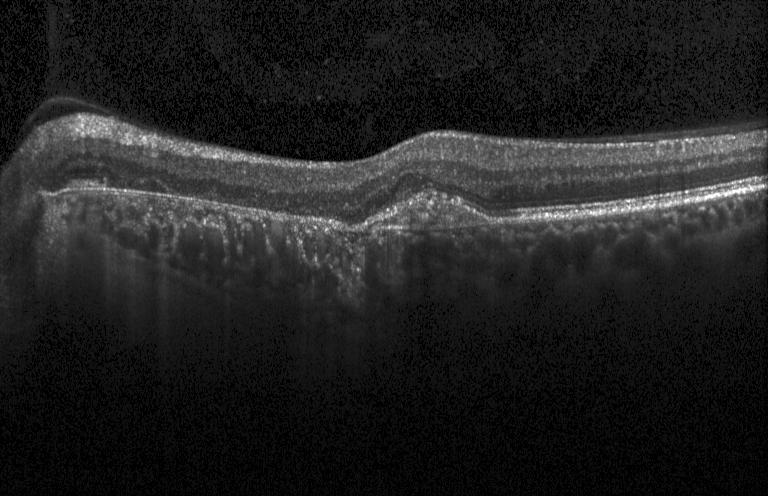 Spectral-domain optical coherence tomography · optical coherence tomography scan · Heidelberg Spectralis · fovea-centered.
Finding: a choroidal neovascular membrane.